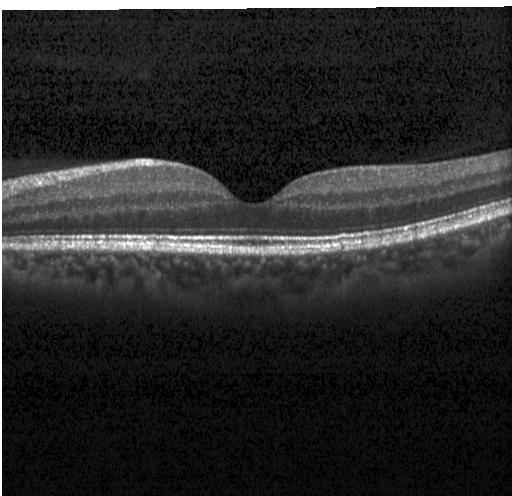
OCT B-scan. Assessment: neither CNV, DME, nor drusen.